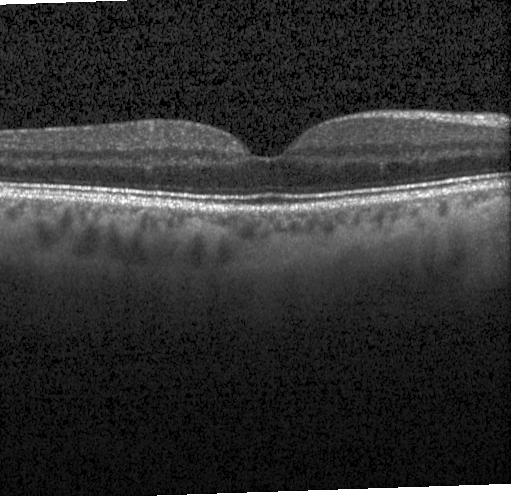

OCT B-scan
Finding: no choroidal neovascularization, diabetic macular edema, or drusen.